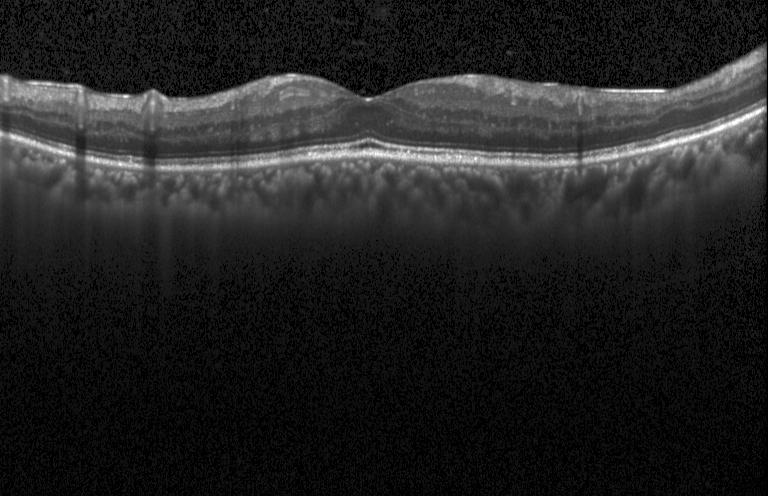

Impression: no choroidal neovascularization, no diabetic macular edema, and no drusen.